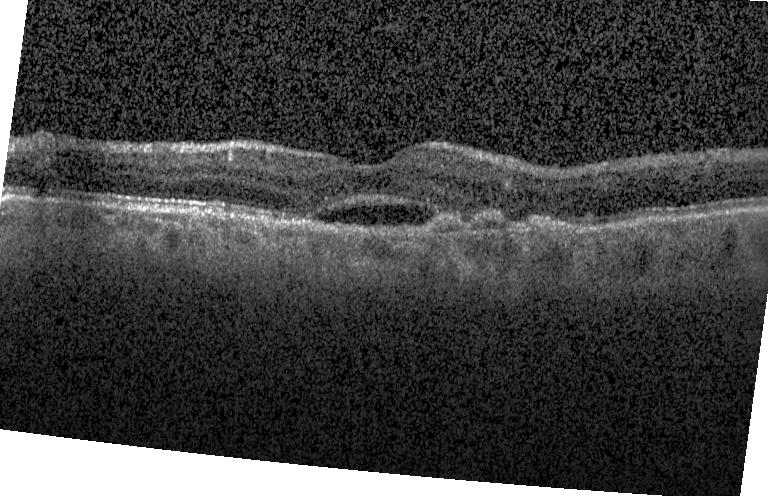 OCT line scan. Horizontal scan through the fovea — Diagnosis: a choroidal neovascular membrane.